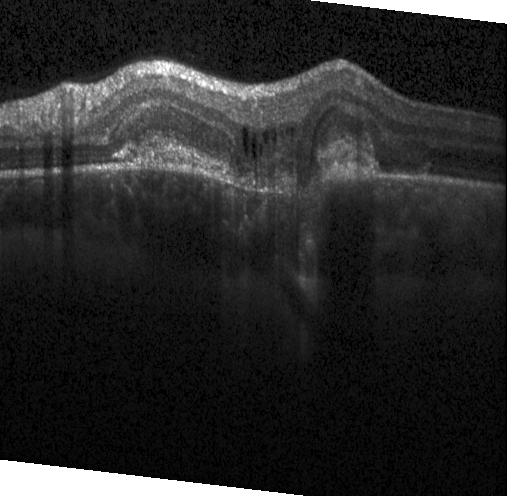

Impression: CNV.